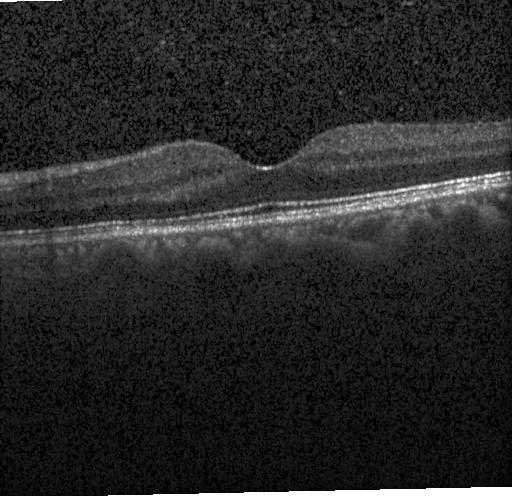
OCT line scan — Impression: no evidence of CNV, DME, or drusen.